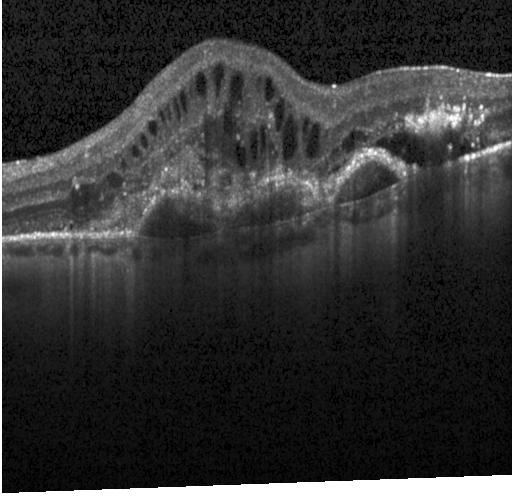
Acquired on a Heidelberg Spectralis. Horizontal scan through the fovea. SD-OCT. OCT line scan — The scan shows choroidal neovascularization (CNV).